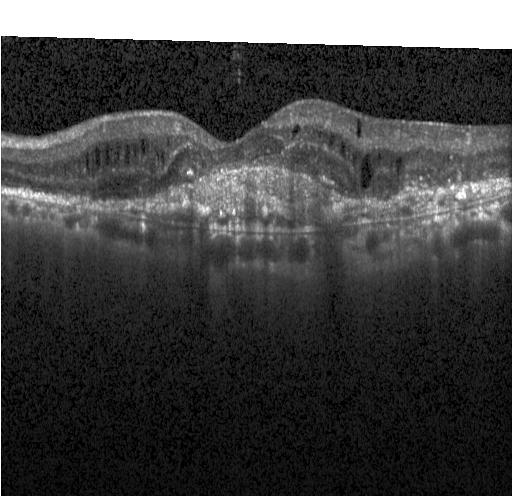
Macular OCT: a choroidal neovascular membrane.